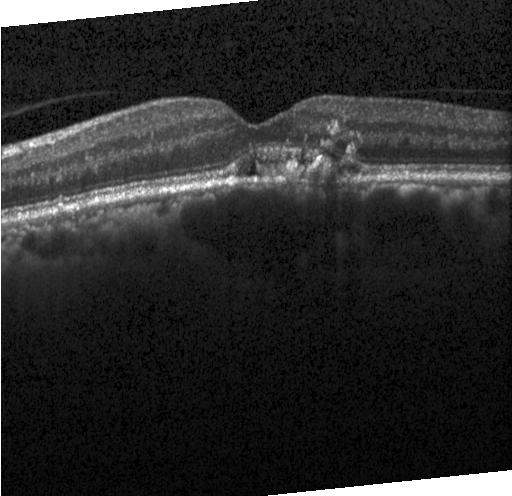

Acquired on a Heidelberg Spectralis; SD-OCT; OCT B-scan
Diagnosis: choroidal neovascularization.